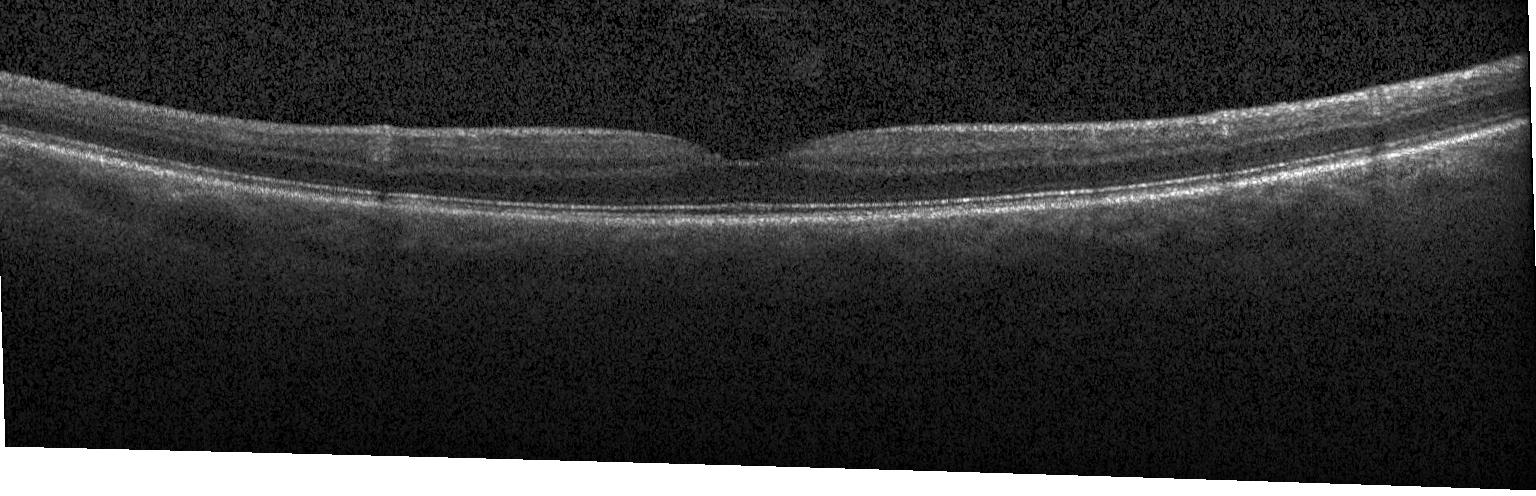
Macular OCT: no CNV, no DME, and no drusen.